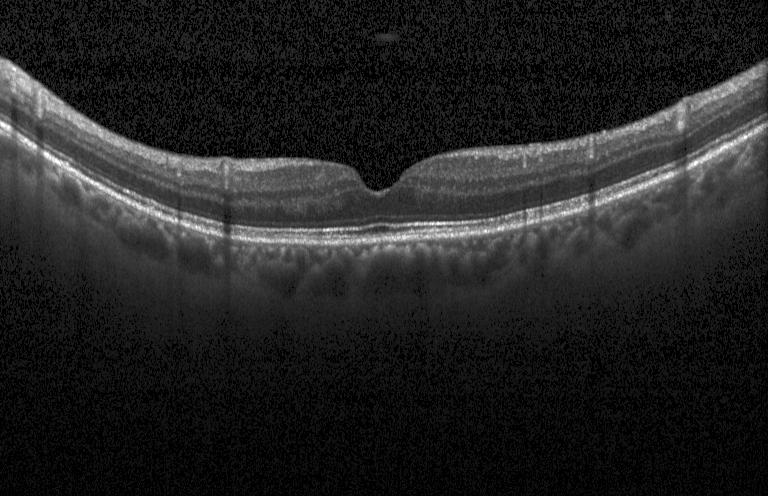
Spectral-domain optical coherence tomography · acquired on a Heidelberg Spectralis · retinal OCT cross-section. Finding: no evidence of choroidal neovascularization, diabetic macular edema, or drusen.